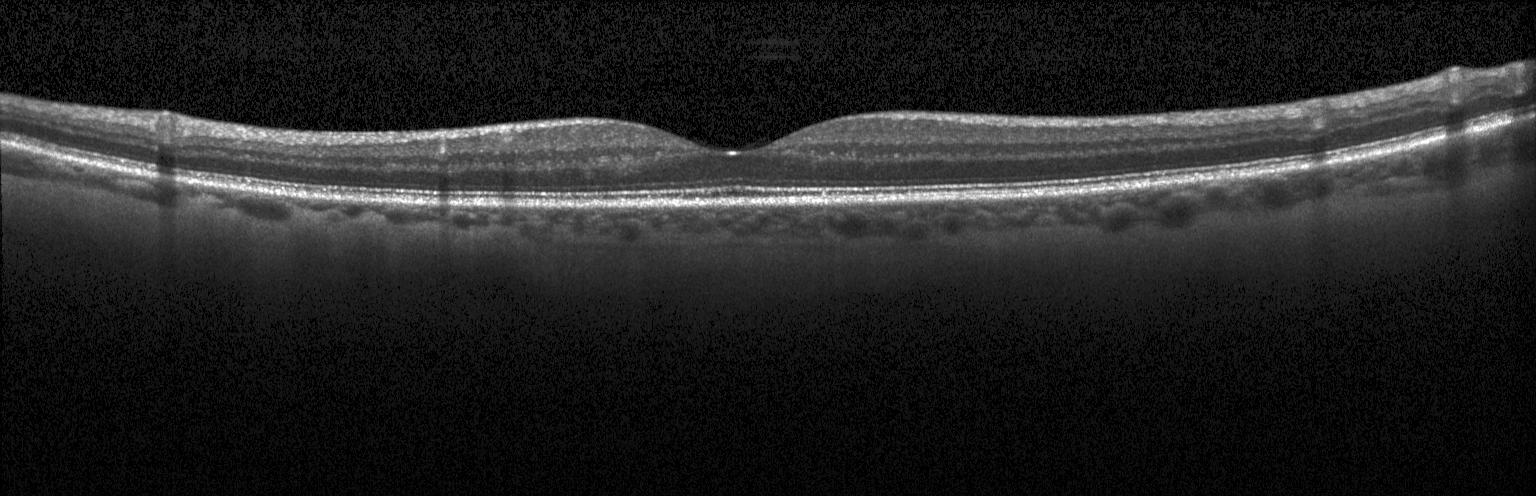

SD-OCT; macular scan; optical coherence tomography scan. Finding: no CNV, DME, or drusen.